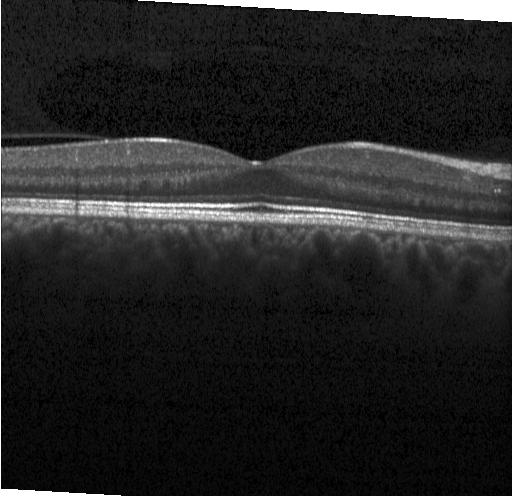 Retinal OCT B-scan.
Diagnosis: no evidence of CNV, DME, or drusen.